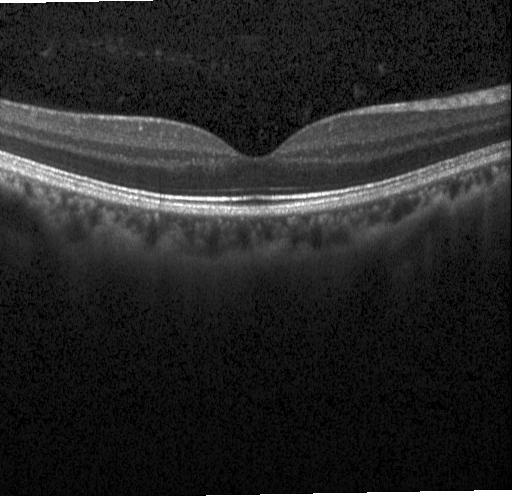 SD-OCT; macular scan; optical coherence tomography B-scan; acquired on a Heidelberg Spectralis.
Diagnosis: no choroidal neovascularization, diabetic macular edema, or drusen.